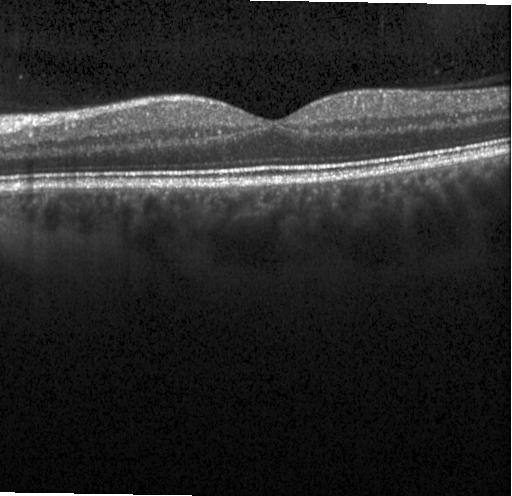

Retinal OCT cross-section
Assessment: no choroidal neovascularization, no diabetic macular edema, and no drusen.